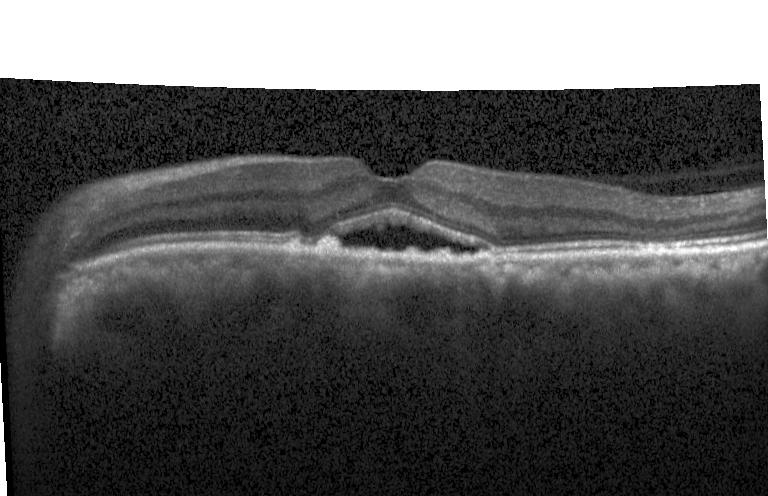 Dx: choroidal neovascularization (CNV).